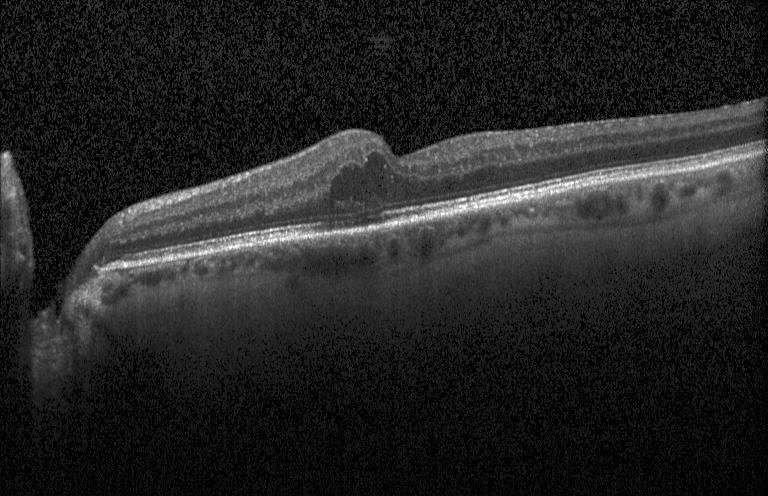 Dx: DME.